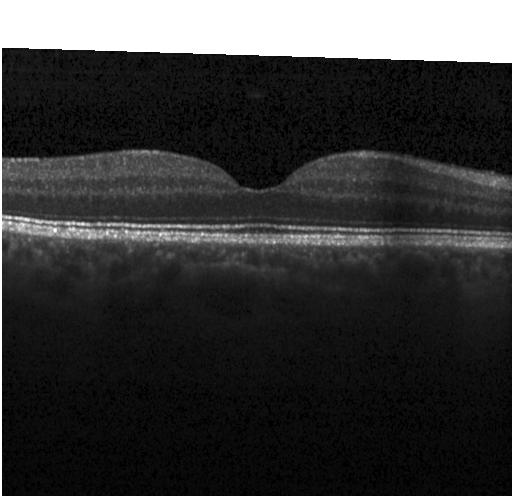 Instrument: Heidelberg Spectralis, spectral-domain OCT, optical coherence tomography B-scan.
Impression: no choroidal neovascularization, diabetic macular edema, or drusen.